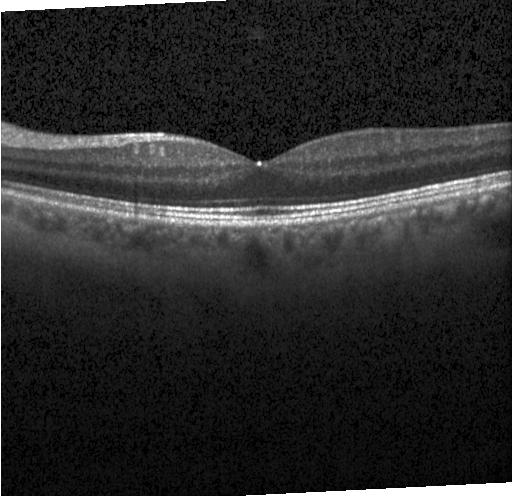

Through the macula. Optical coherence tomography scan. Heidelberg Spectralis OCT system — Assessment: neither choroidal neovascularization, diabetic macular edema, nor drusen.